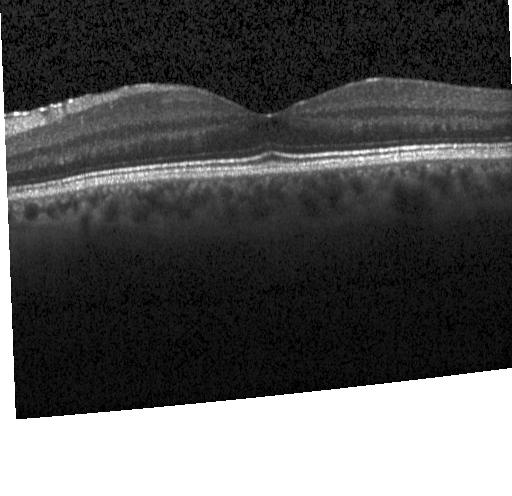 Macular scan · Heidelberg Spectralis OCT system · OCT line scan — Diagnosis: no choroidal neovascularization, no diabetic macular edema, and no drusen.